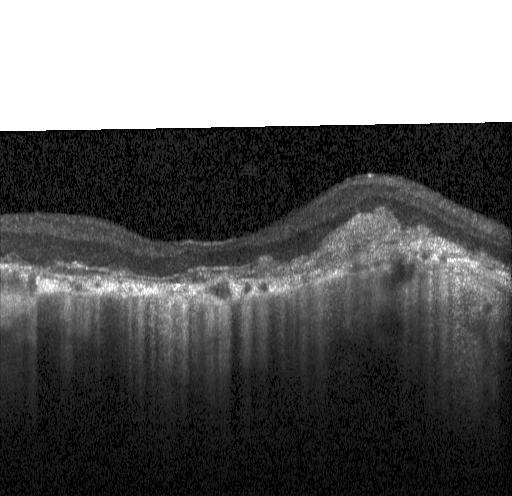

Macular scan, retinal OCT B-scan, acquired on a Heidelberg Spectralis, SD-OCT — Macular OCT: choroidal neovascularization.